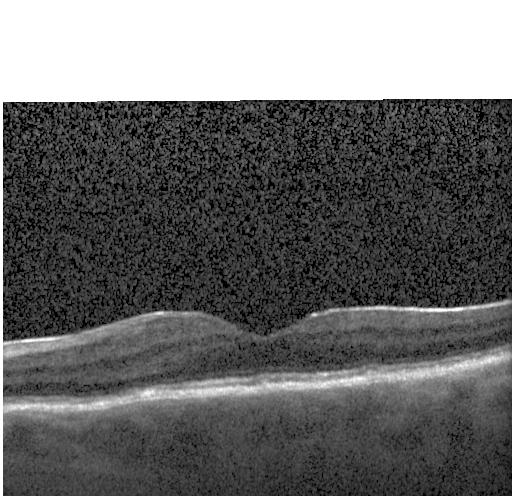
OCT B-scan. Impression: no choroidal neovascularization, diabetic macular edema, or drusen.